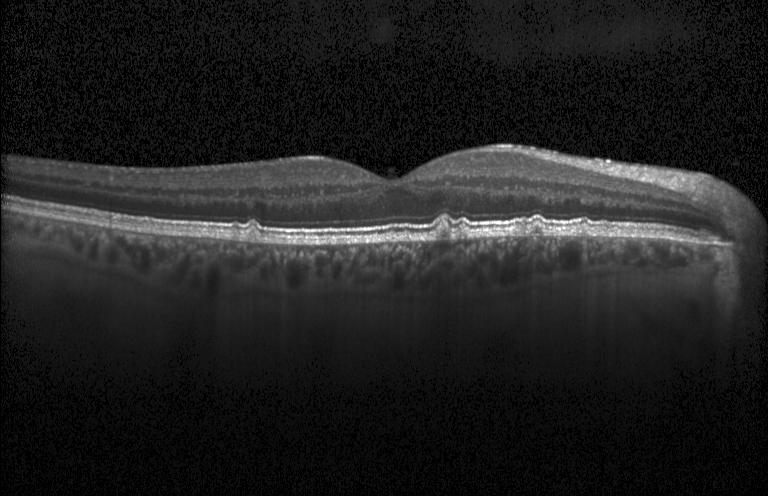 Spectral-domain OCT · retinal OCT B-scan · Heidelberg Spectralis OCT system
Diagnosis: drusen.